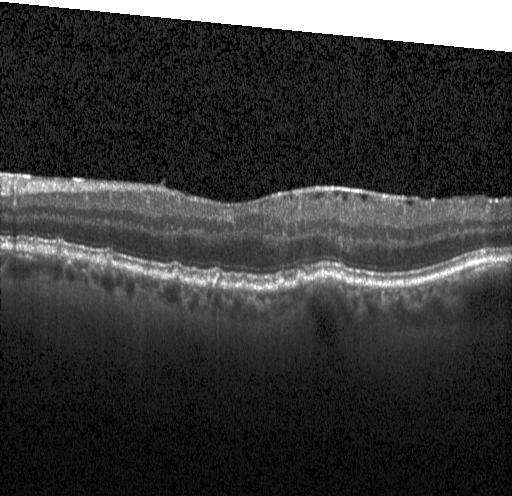

Optical coherence tomography B-scan, Heidelberg Spectralis, centered on the fovea, spectral-domain OCT.
Diagnosis: multiple drusen.